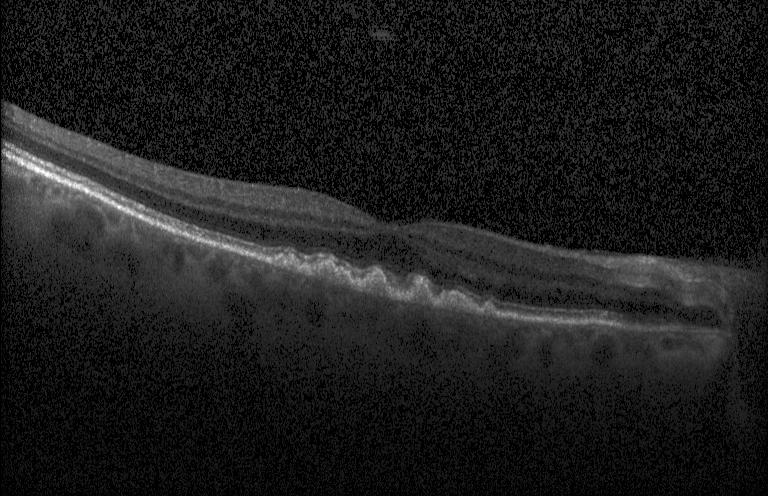

Retinal OCT B-scan. Diagnosis: sub-RPE drusenoid deposits.